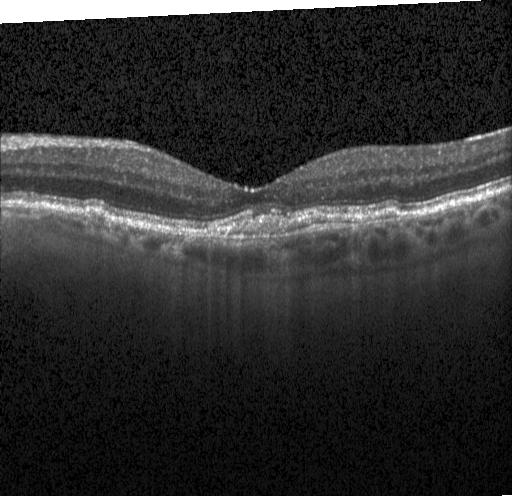

This B-scan demonstrates CNV.